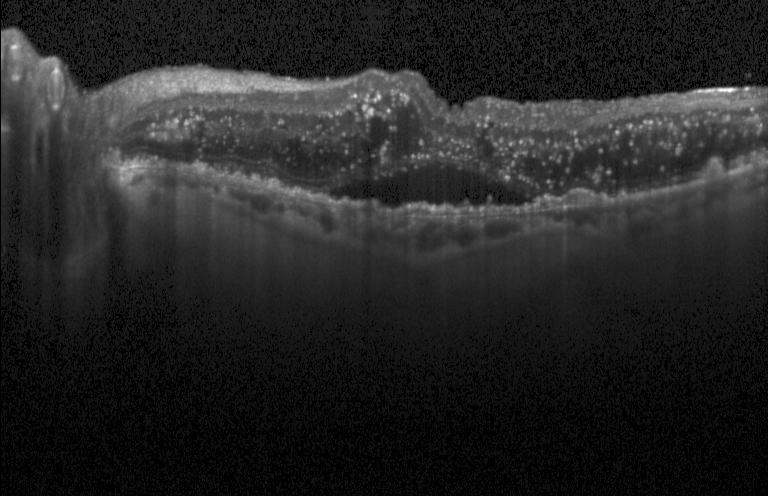
Instrument: Heidelberg Spectralis · macular scan · optical coherence tomography scan · spectral-domain optical coherence tomography — Diagnosis: a choroidal neovascular membrane.